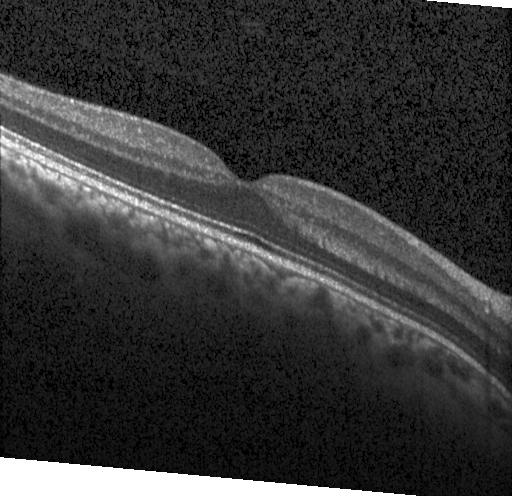
Optical coherence tomography B-scan; acquired on a Heidelberg Spectralis; spectral-domain optical coherence tomography. Macular OCT: no evidence of choroidal neovascularization, diabetic macular edema, or drusen.